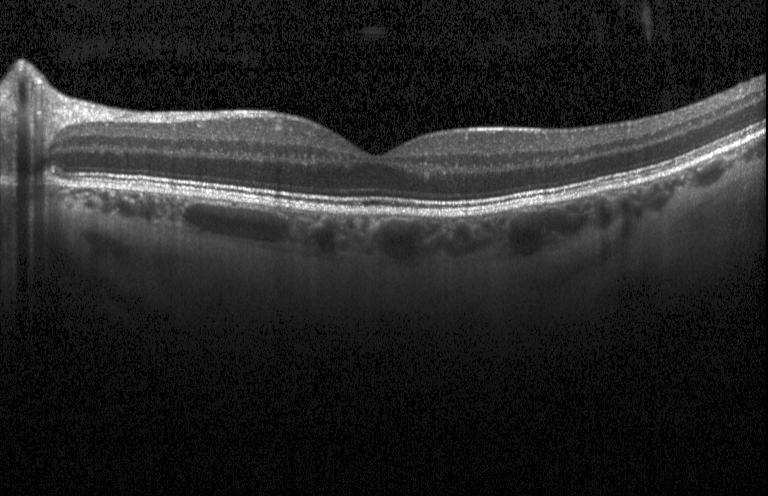 Optical coherence tomography B-scan, spectral-domain optical coherence tomography.
No evidence of choroidal neovascularization, diabetic macular edema, or drusen.